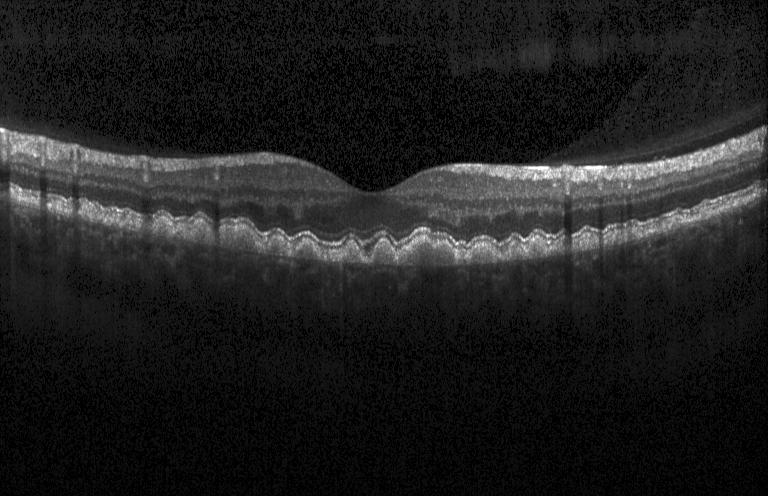 Impression: drusen.